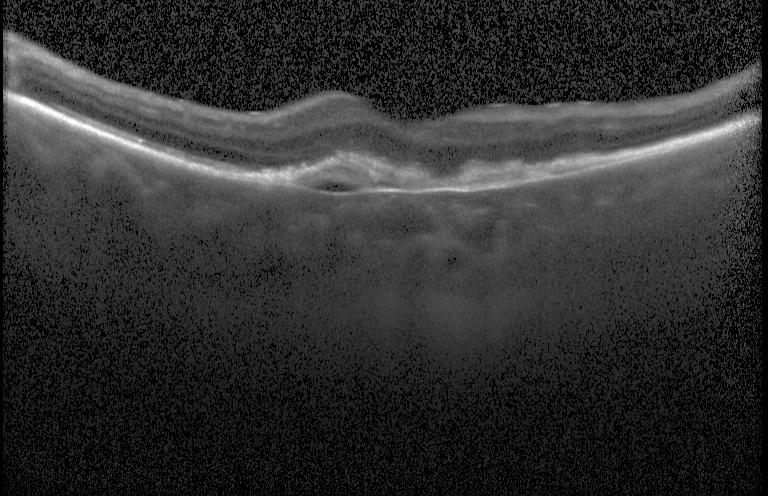
Optical coherence tomography scan; acquired on a Heidelberg Spectralis; through the macula — This B-scan demonstrates a choroidal neovascular membrane.